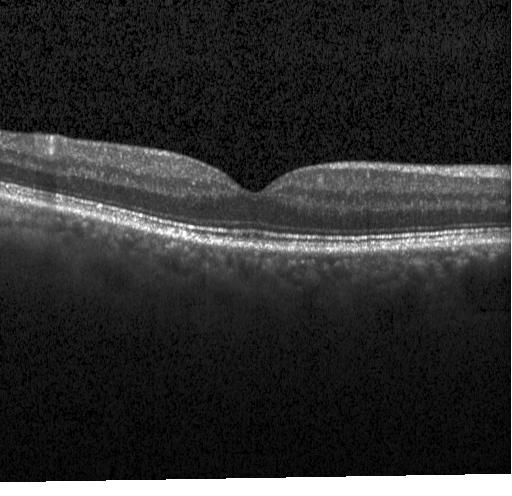
Instrument: Heidelberg Spectralis; fovea-centered; retinal OCT B-scan — The scan shows neither CNV, DME, nor drusen.